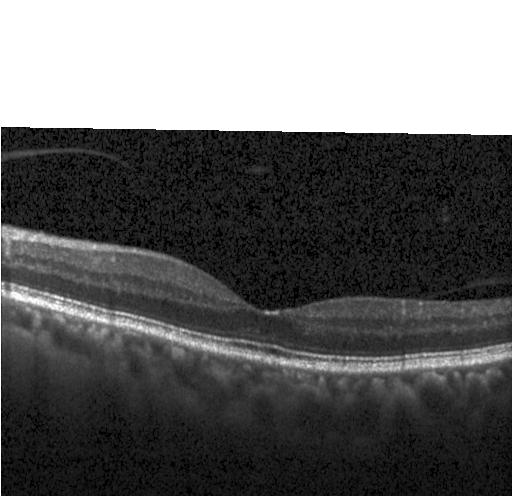 Macular OCT: no choroidal neovascularization, no diabetic macular edema, and no drusen.